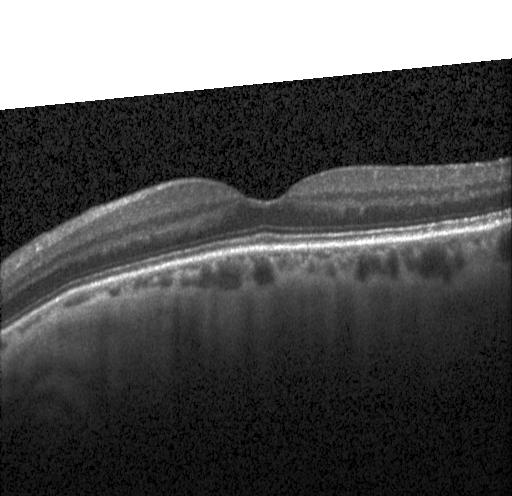

Finding: no evidence of CNV, DME, or drusen.